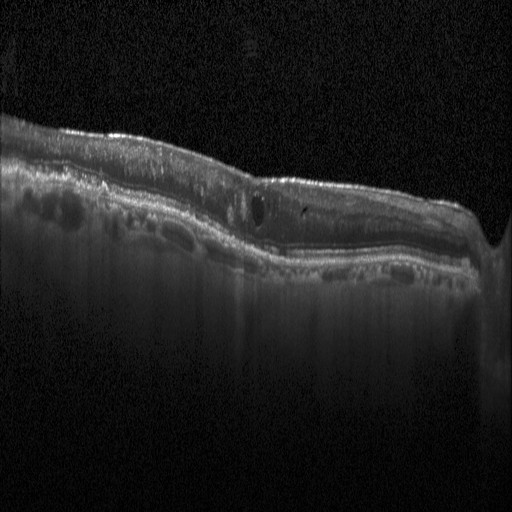 The scan shows diabetic macular edema.